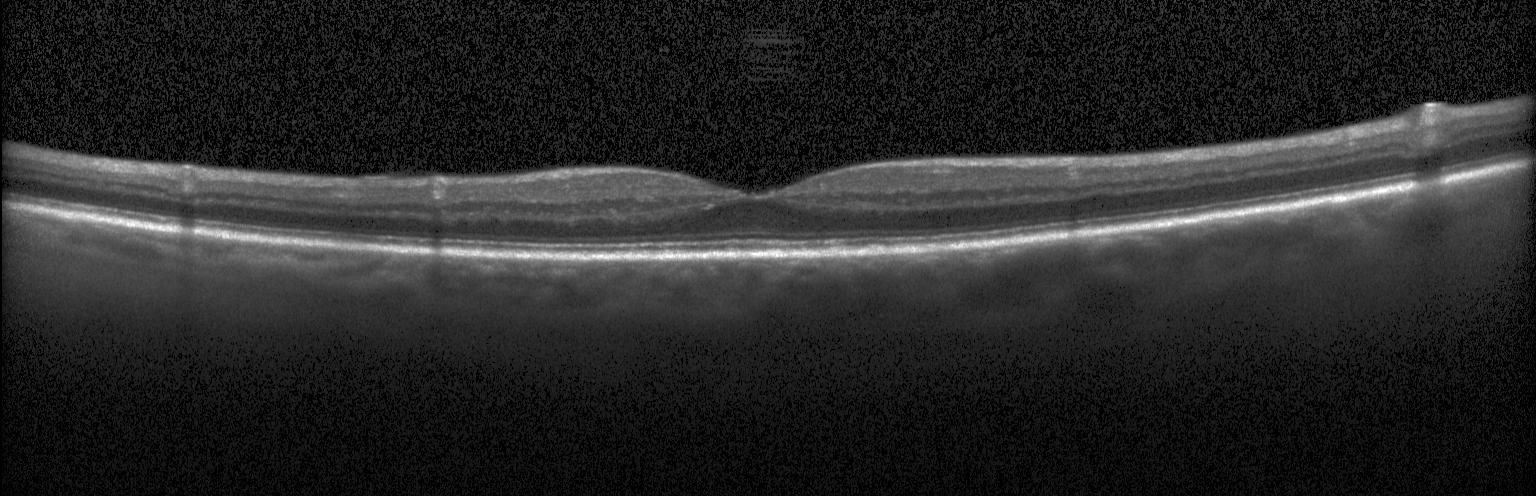 Optical coherence tomography scan, instrument: Heidelberg Spectralis
No CNV, no DME, and no drusen.